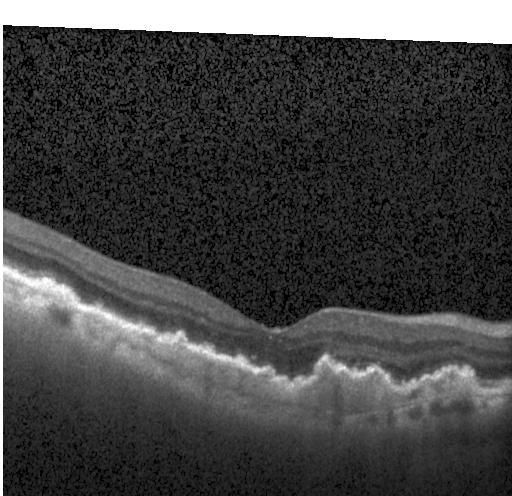 Centered on the fovea · Heidelberg Spectralis OCT system · spectral-domain OCT · retinal OCT B-scan.
Choroidal neovascularization.